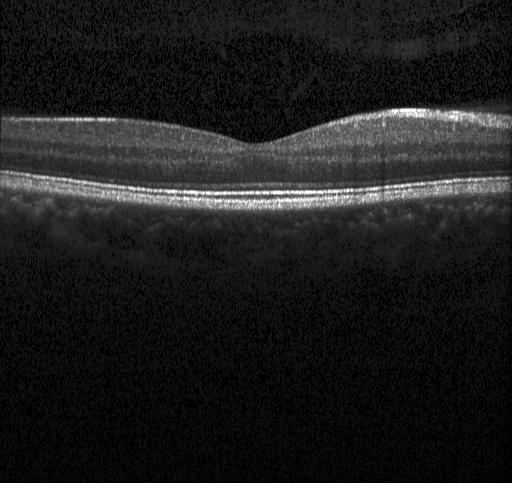
OCT line scan
Finding: neither CNV, DME, nor drusen.